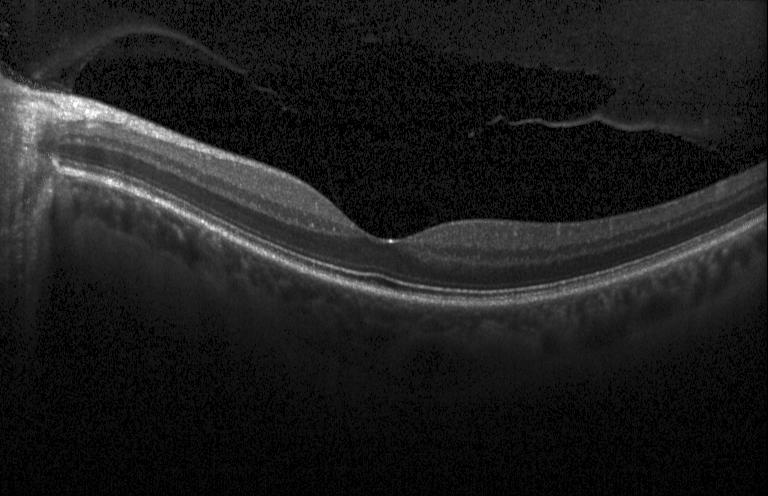

Optical coherence tomography scan
This B-scan demonstrates neither choroidal neovascularization, diabetic macular edema, nor drusen.